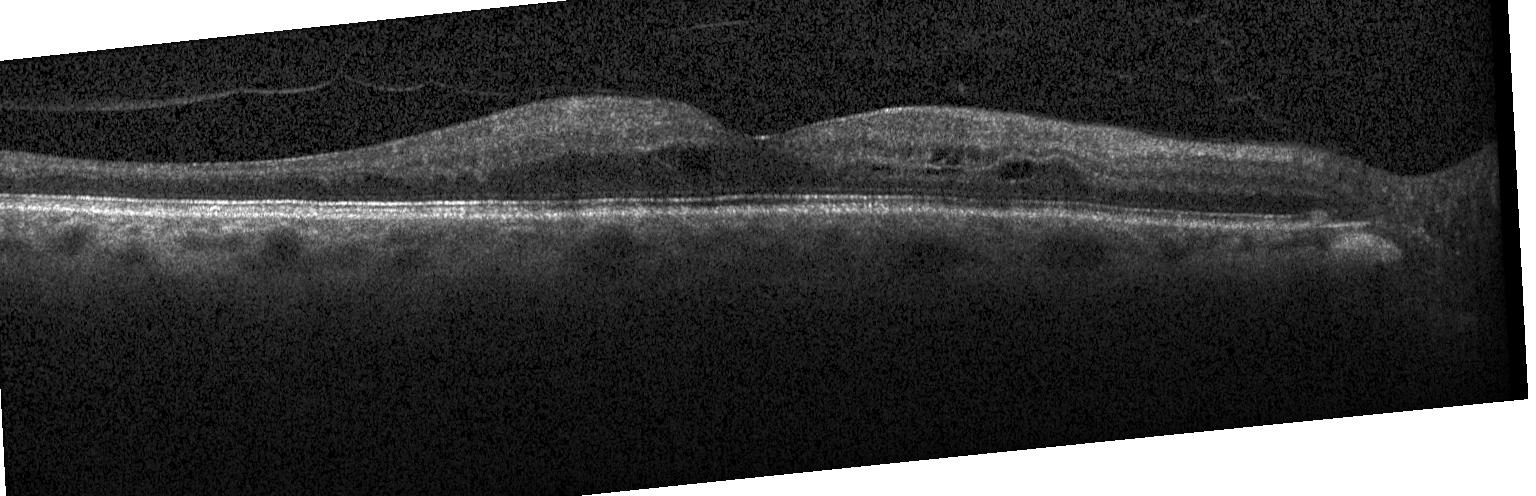

OCT B-scan — Diagnosis: DME.